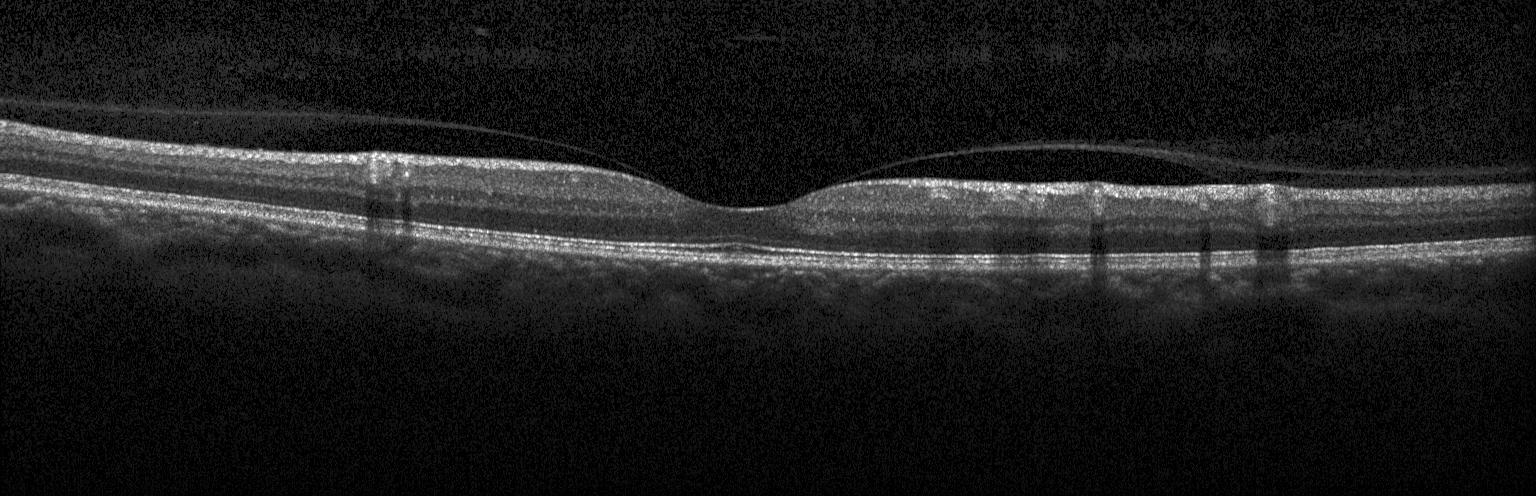
OCT B-scan, spectral-domain optical coherence tomography, through the macula, acquired on a Heidelberg Spectralis.
This B-scan demonstrates no evidence of choroidal neovascularization, diabetic macular edema, or drusen.